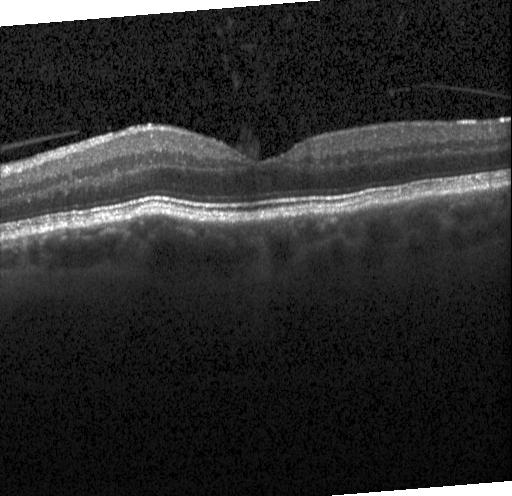 Spectral-domain OCT; OCT line scan.
Finding: no CNV, no DME, and no drusen.